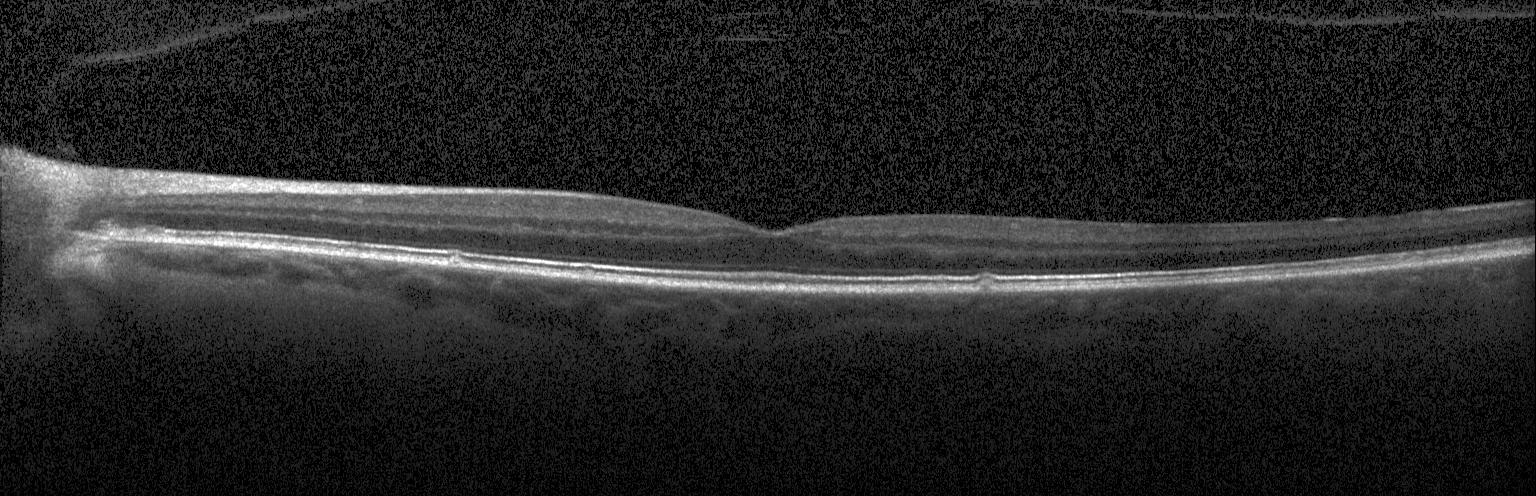

Retinal OCT cross-section
Diagnosis: multiple drusen.